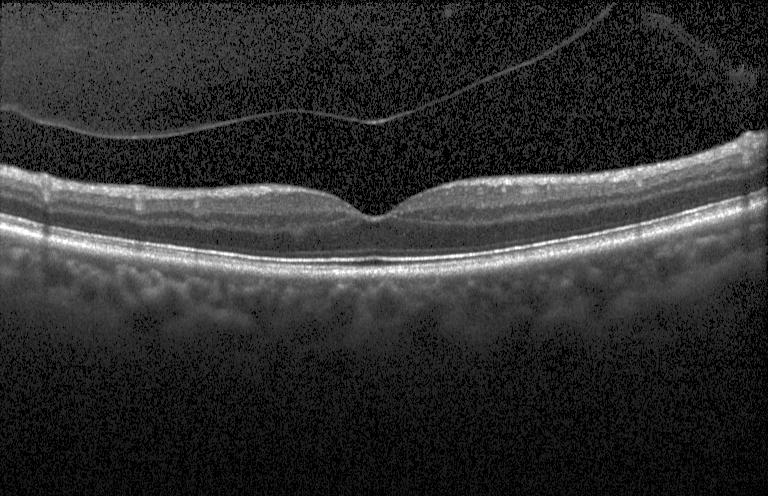 Macular OCT demonstrating no evidence of choroidal neovascularization, diabetic macular edema, or drusen.